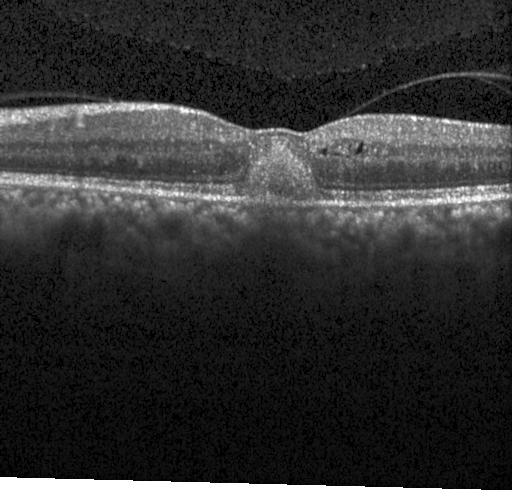 This B-scan demonstrates a choroidal neovascular membrane.